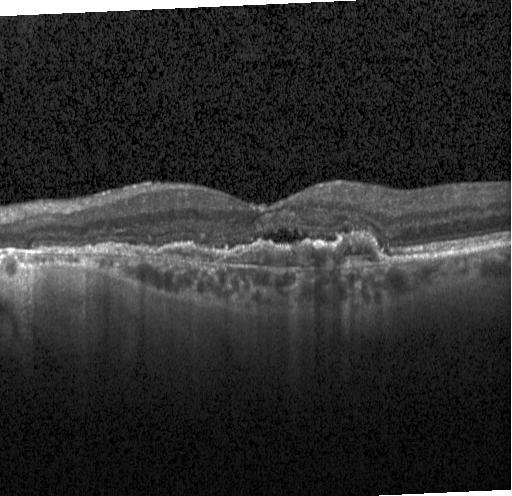
OCT B-scan
Diagnosis: a choroidal neovascular membrane.